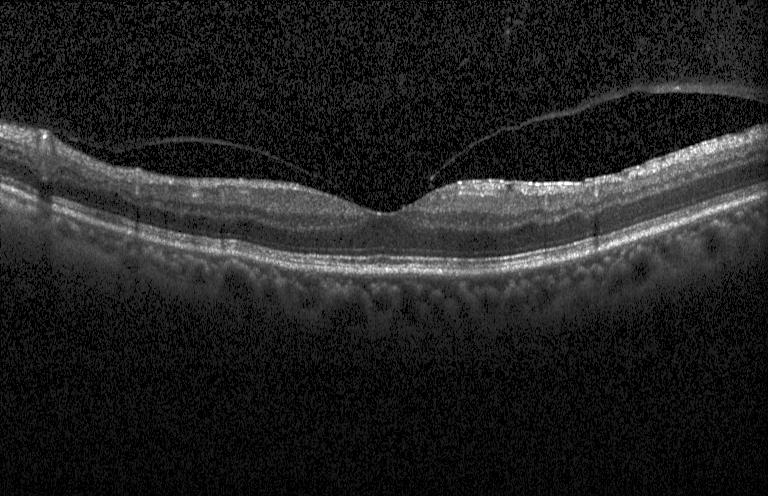 Dx: neither choroidal neovascularization, diabetic macular edema, nor drusen.